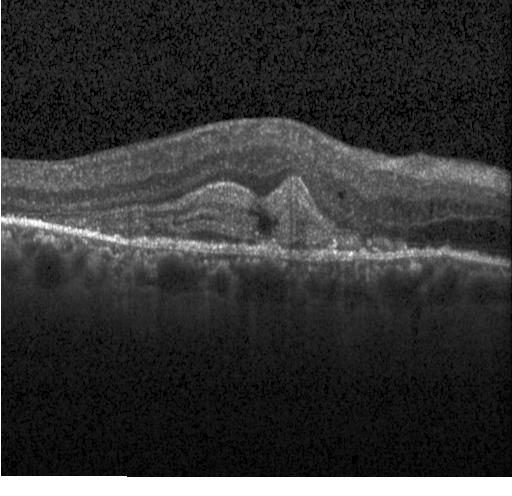
Optical coherence tomography B-scan
Assessment: a choroidal neovascular membrane.